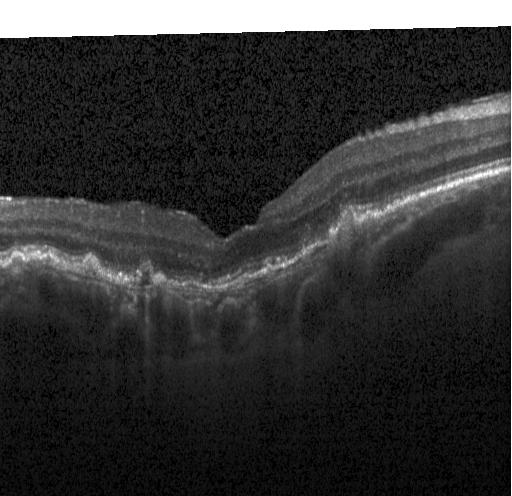 Spectral-domain optical coherence tomography · macular scan · instrument: Heidelberg Spectralis · optical coherence tomography scan
Impression: a choroidal neovascular membrane.